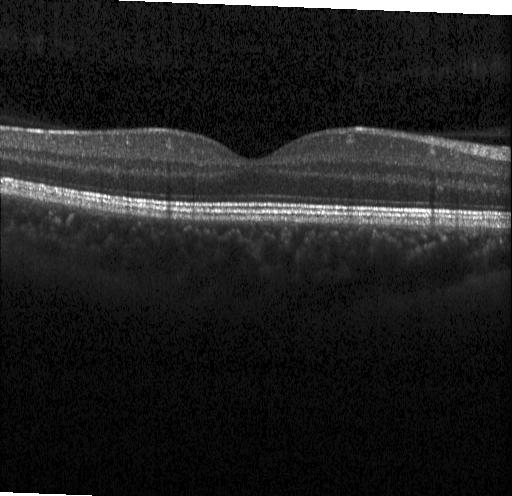

OCT line scan. Macular OCT: neither choroidal neovascularization, diabetic macular edema, nor drusen.